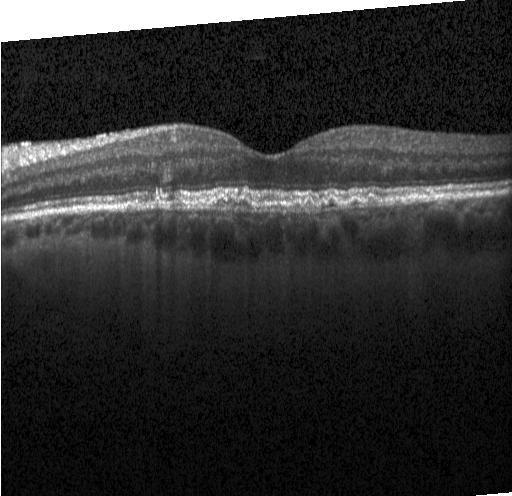 Retinal OCT cross-section. Instrument: Heidelberg Spectralis. SD-OCT. Through the macula
Sub-RPE drusenoid deposits.